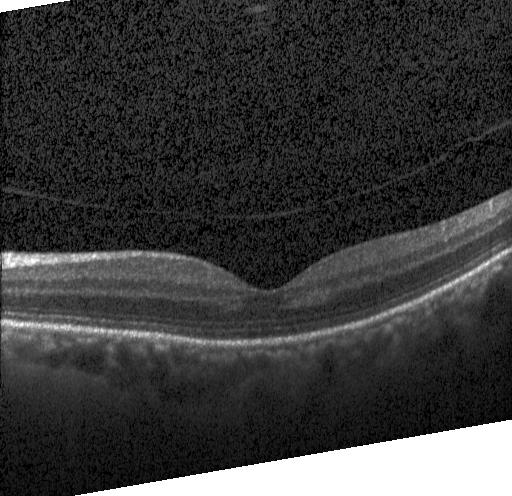
The scan shows no choroidal neovascularization, diabetic macular edema, or drusen.